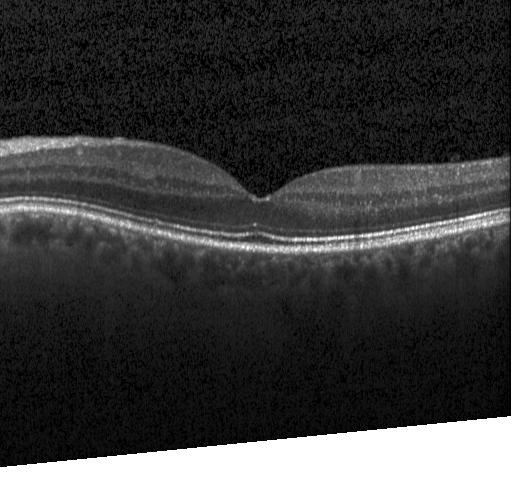

Through the macula; spectral-domain optical coherence tomography; OCT B-scan.
The scan shows neither CNV, DME, nor drusen.